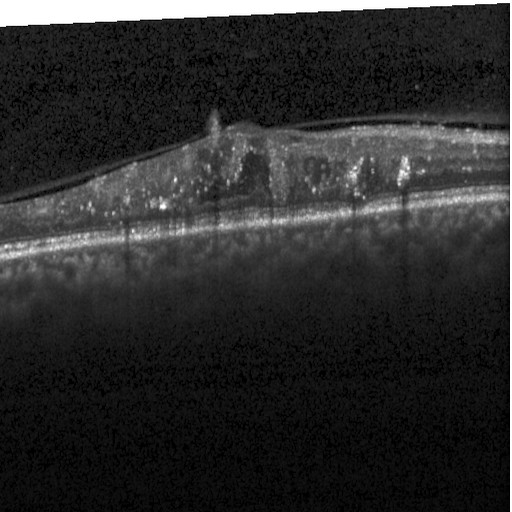

Retinal OCT cross-section, spectral-domain OCT.
Finding: diabetic macular edema.